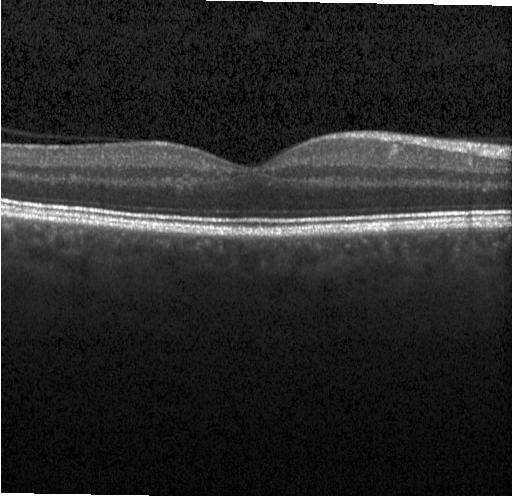

Impression: neither CNV, DME, nor drusen.